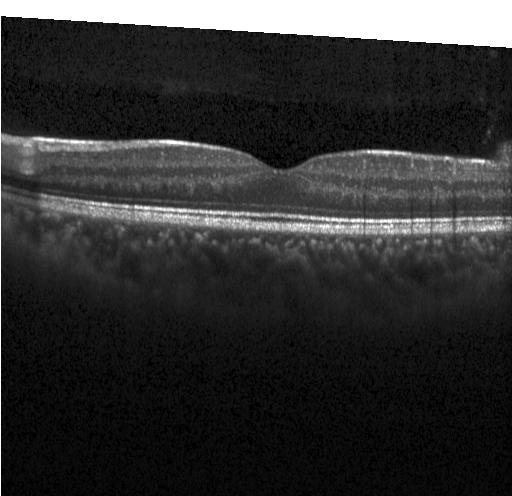
Finding: no choroidal neovascularization, diabetic macular edema, or drusen.